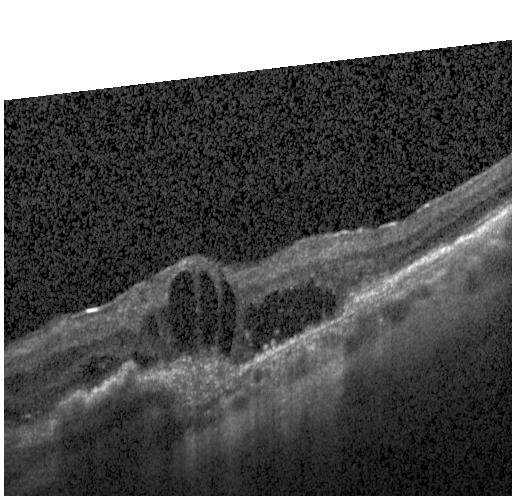
Macular OCT: CNV.